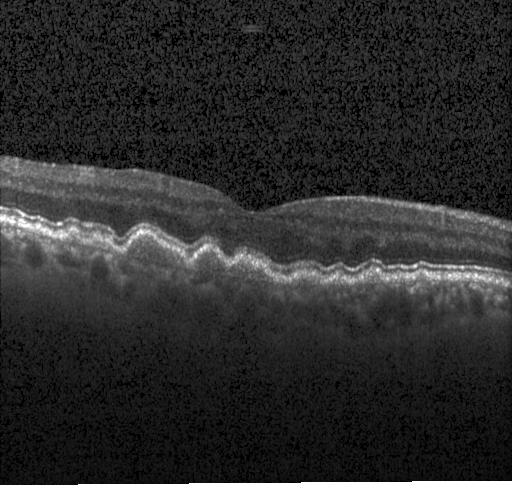

OCT B-scan showing multiple drusen.